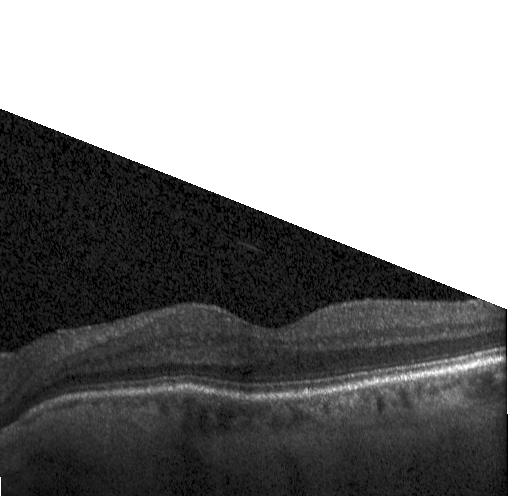 Retinal OCT B-scan.
This B-scan demonstrates no choroidal neovascularization, diabetic macular edema, or drusen.